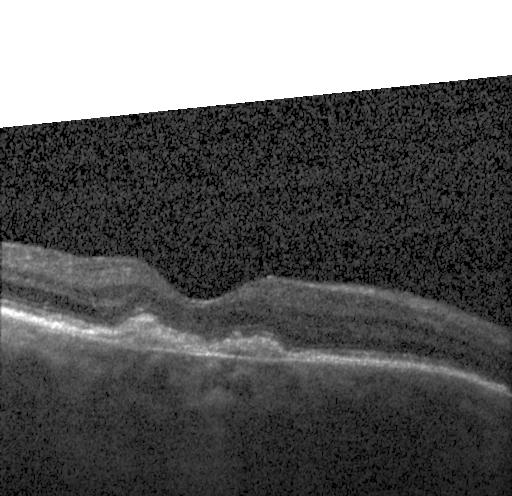 The scan shows CNV.